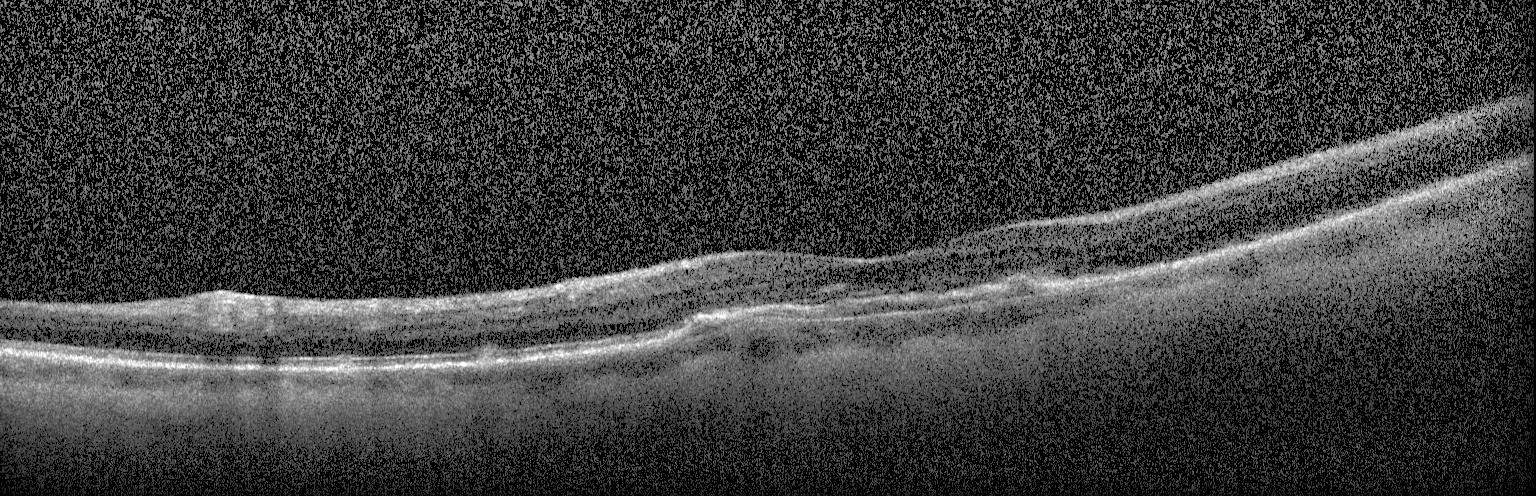 OCT line scan. Assessment: a choroidal neovascular membrane.